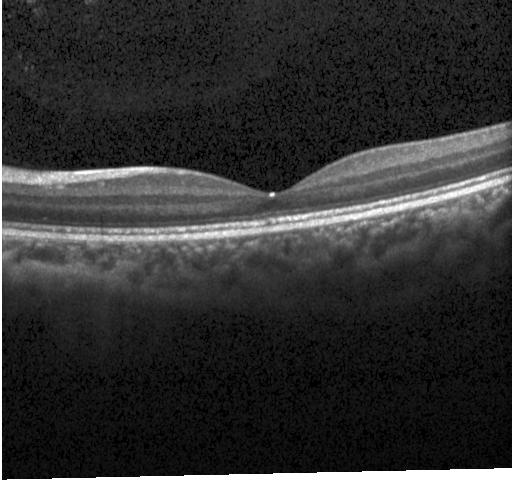

OCT finding: no CNV, no DME, and no drusen.